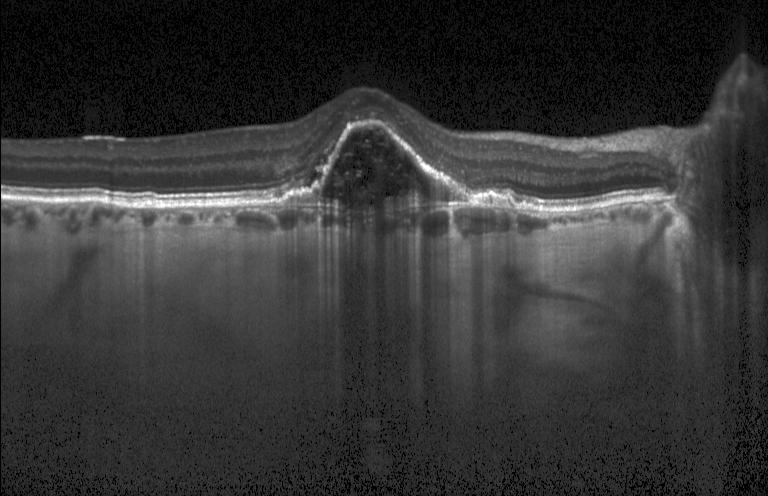
Finding: choroidal neovascularization.